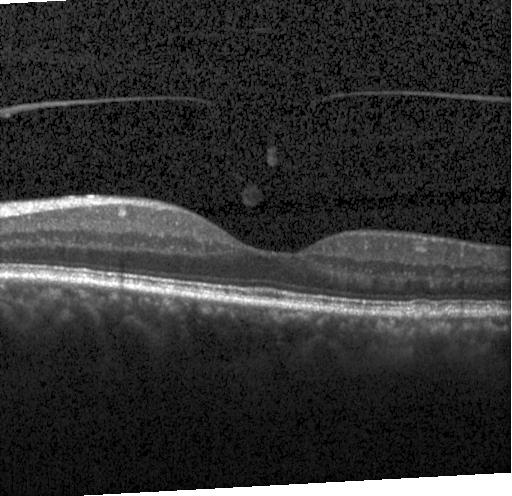

Instrument: Heidelberg Spectralis. Retinal OCT cross-section. This B-scan demonstrates no choroidal neovascularization, diabetic macular edema, or drusen.